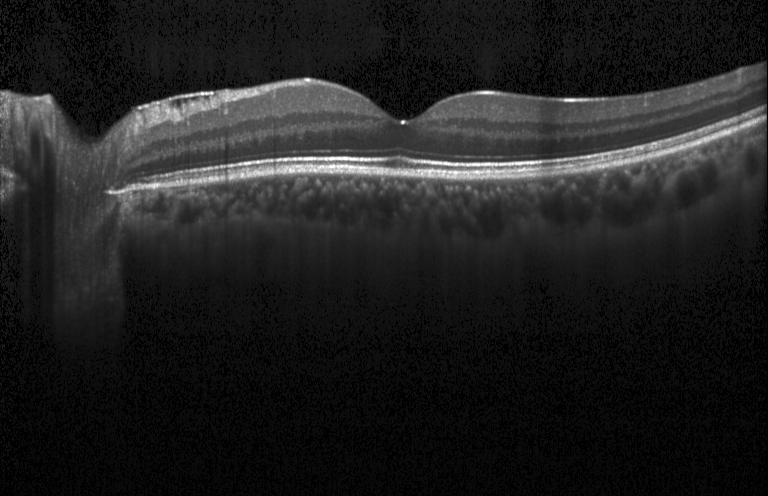

Heidelberg Spectralis. Fovea-centered. OCT line scan — Finding: no evidence of CNV, DME, or drusen.